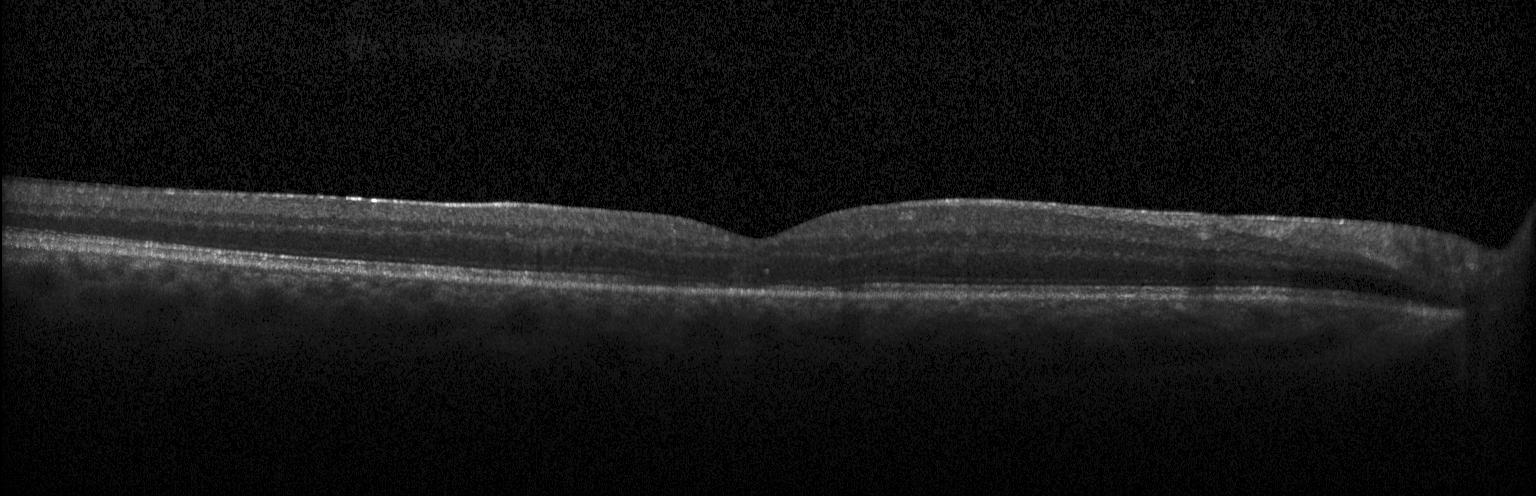 Optical coherence tomography scan. Diagnosis: no choroidal neovascularization, no diabetic macular edema, and no drusen.